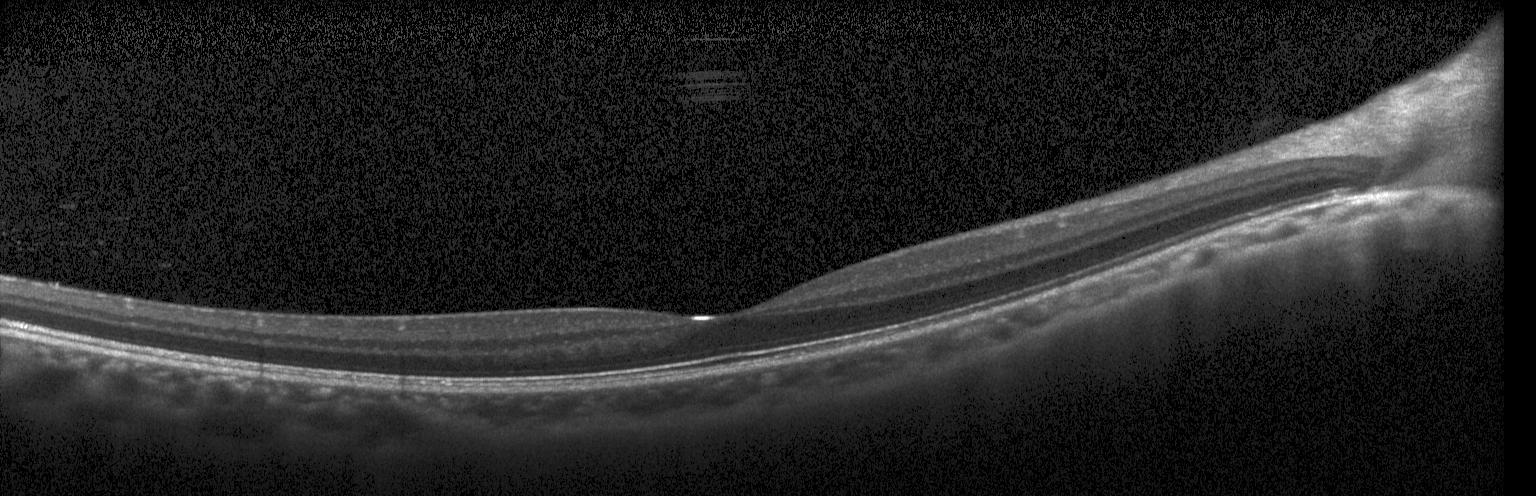

Dx: neither CNV, DME, nor drusen.